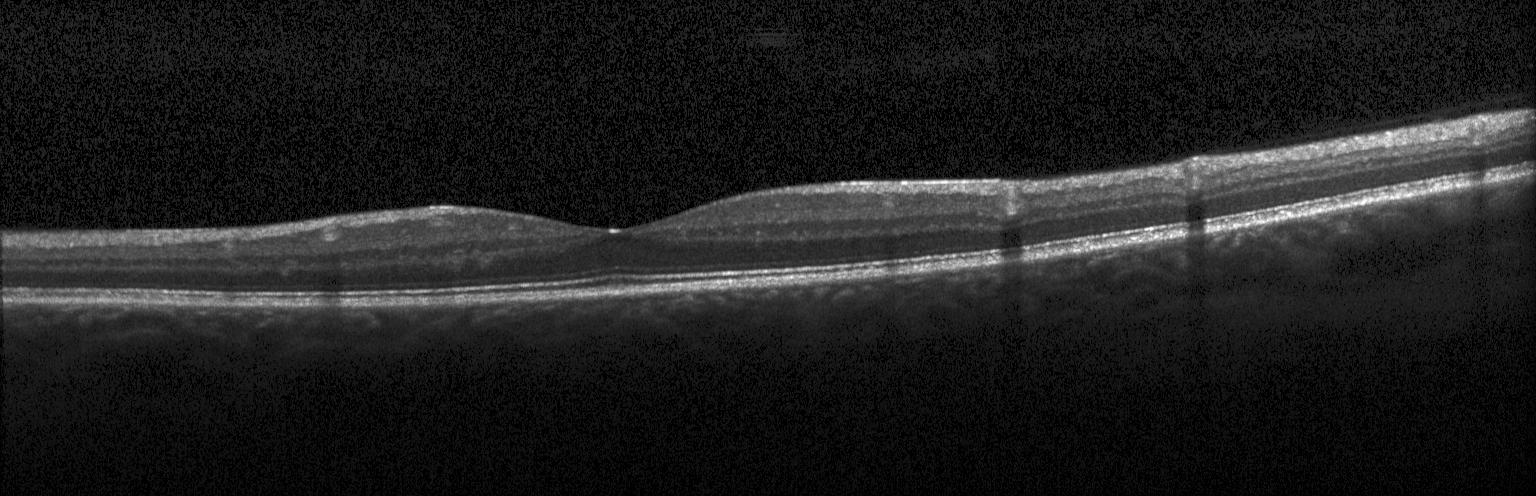
OCT B-scan; acquired on a Heidelberg Spectralis. Neither CNV, DME, nor drusen.